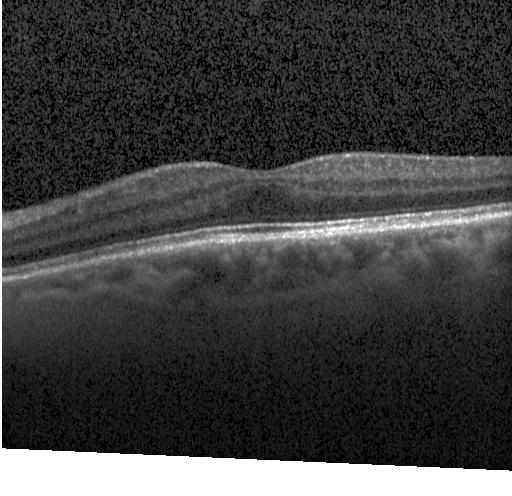
OCT B-scan. SD-OCT. Macular scan. Heidelberg Spectralis OCT system
Macular OCT: no CNV, DME, or drusen.